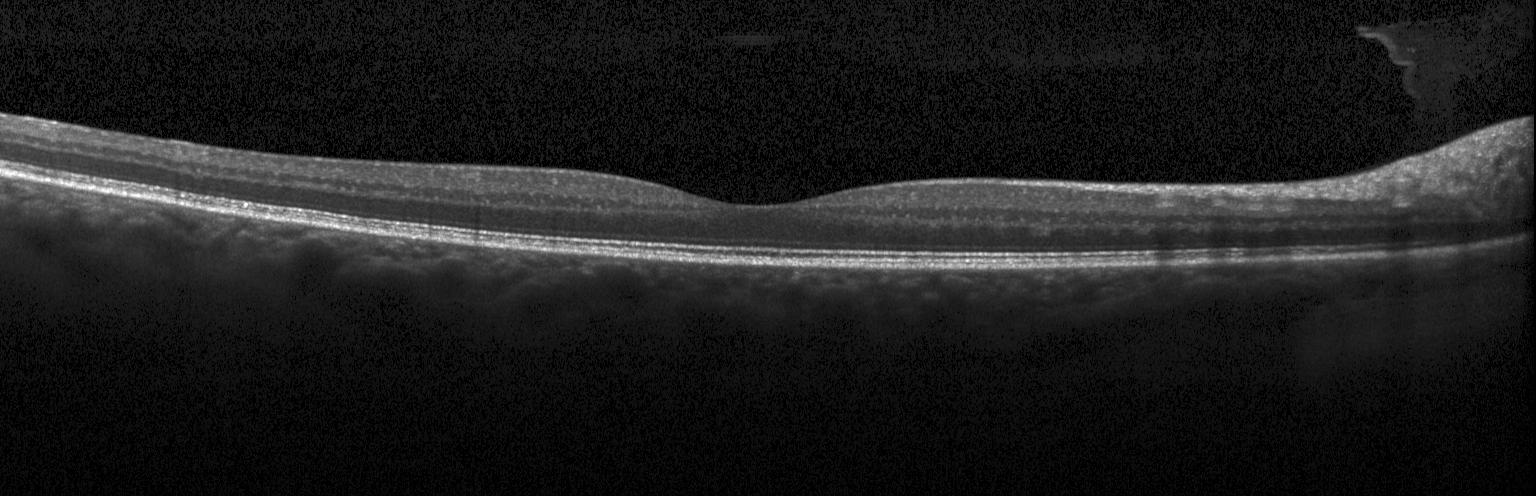 Impression: neither choroidal neovascularization, diabetic macular edema, nor drusen.